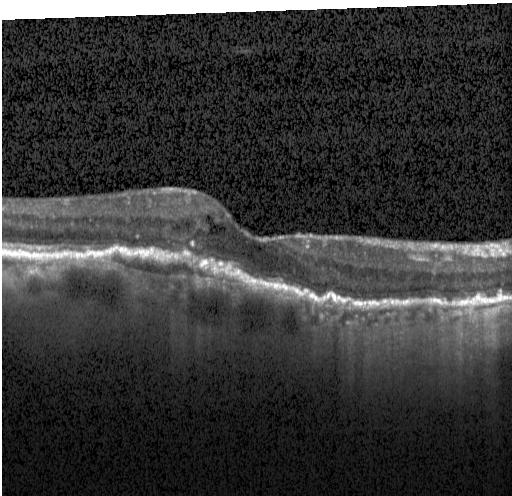 Instrument: Heidelberg Spectralis; optical coherence tomography scan.
Diagnosis: CNV.